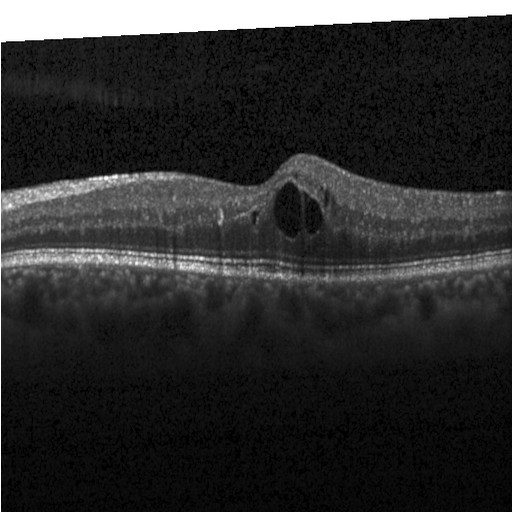 Macular scan, OCT line scan, spectral-domain OCT. Diagnosis: DME.